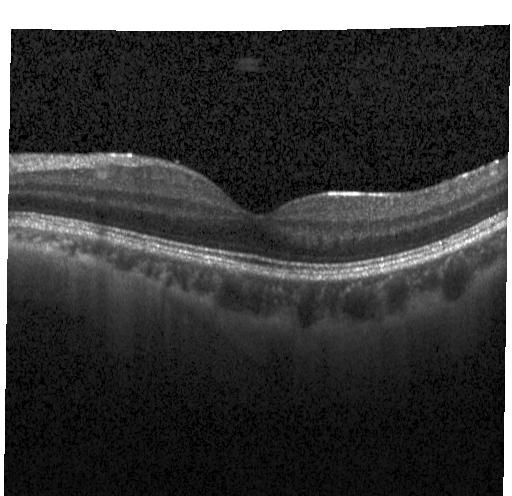
OCT line scan · SD-OCT · instrument: Heidelberg Spectralis · fovea-centered. Impression: no CNV, DME, or drusen.